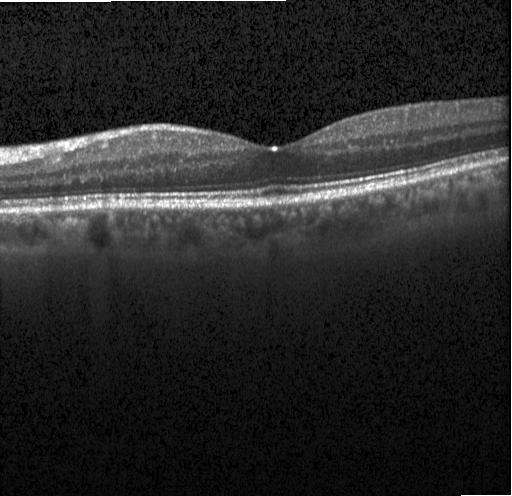 Finding: neither choroidal neovascularization, diabetic macular edema, nor drusen.